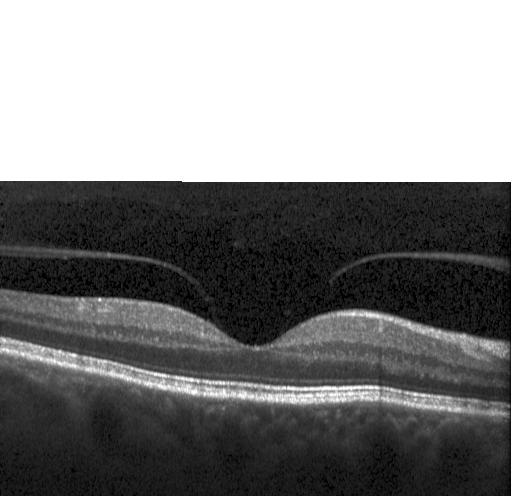

Retinal OCT cross-section, macular scan, acquired on a Heidelberg Spectralis — OCT finding: no choroidal neovascularization, no diabetic macular edema, and no drusen.